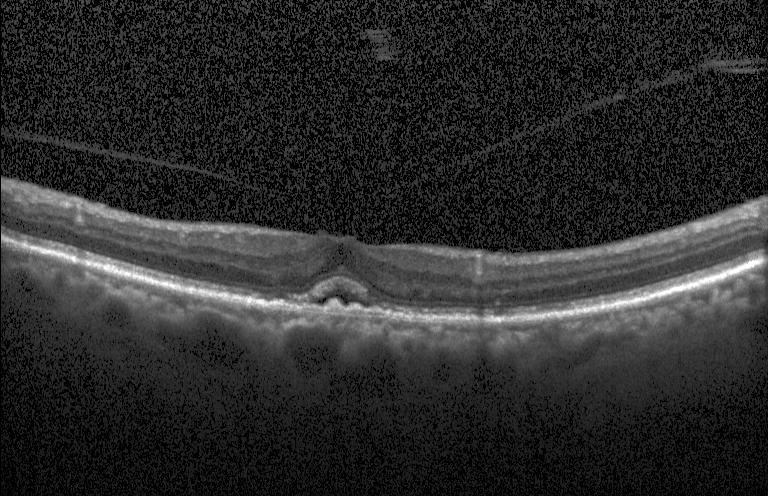 Heidelberg Spectralis OCT system. Optical coherence tomography scan. Fovea-centered — Assessment: CNV.